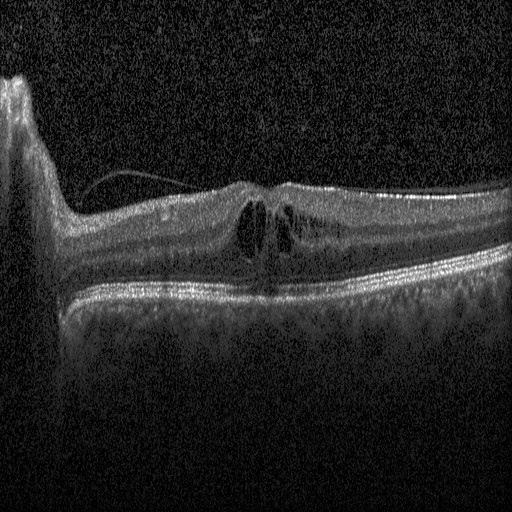 Acquired on a Heidelberg Spectralis · centered on the fovea · optical coherence tomography scan. Impression: diabetic macular edema (DME).